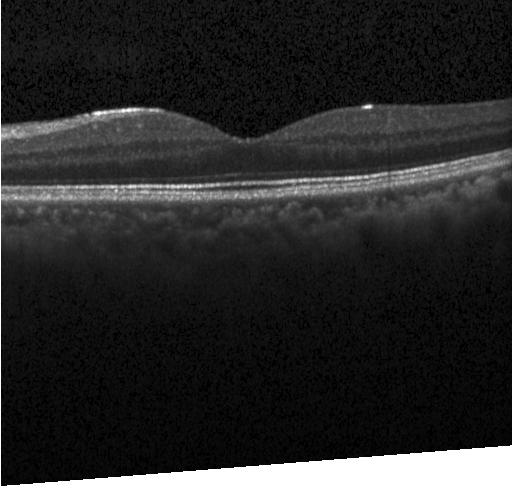
Finding: no evidence of CNV, DME, or drusen.